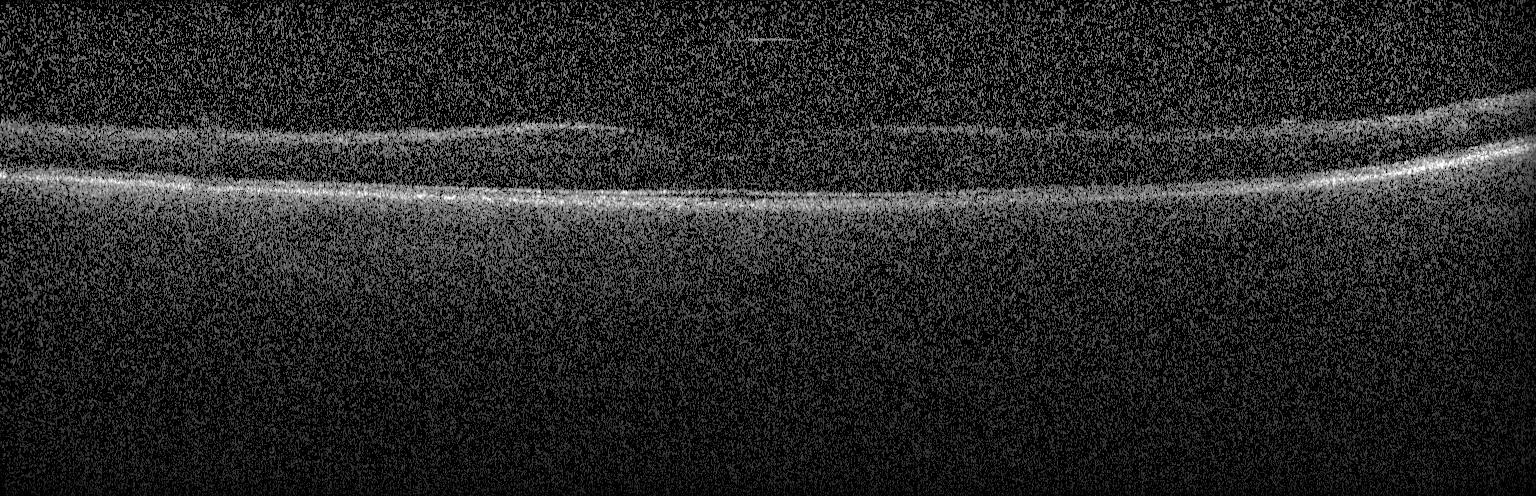 Instrument: Heidelberg Spectralis. Retinal OCT B-scan — Finding: no evidence of choroidal neovascularization, diabetic macular edema, or drusen.